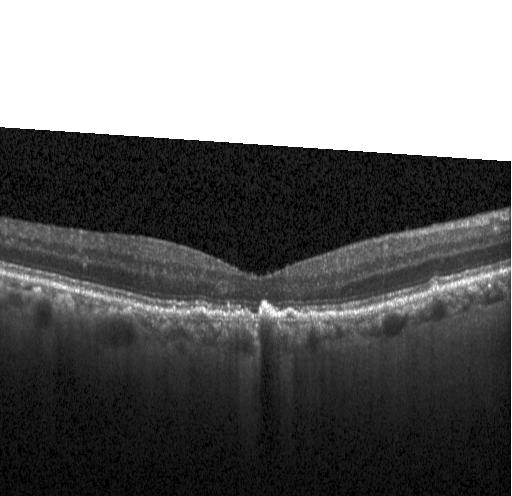

Drusen.